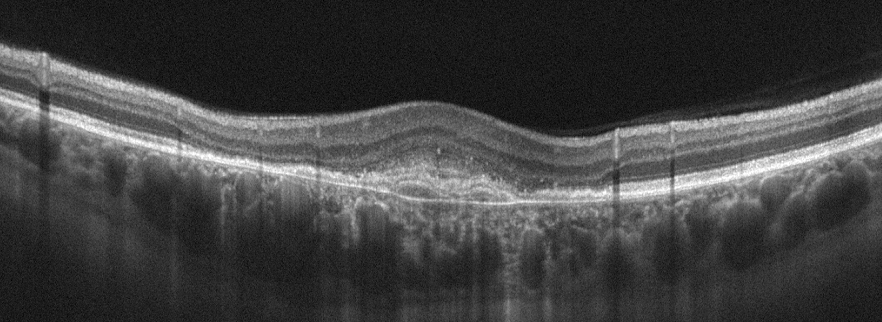

Left eye · optical coherence tomography scan.
Diagnosis: age-related macular degeneration (AMD).